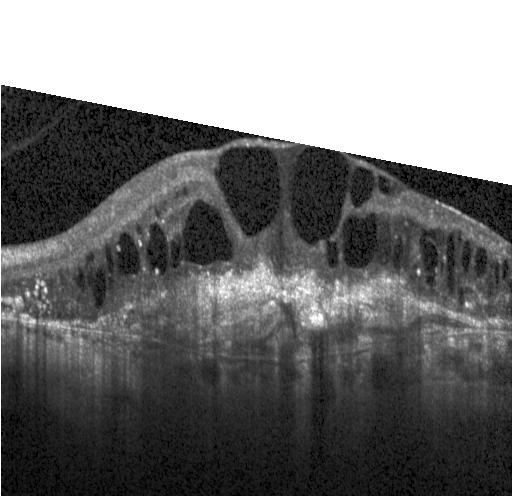
Centered on the fovea; retinal OCT cross-section; acquired on a Heidelberg Spectralis
Impression: choroidal neovascularization.